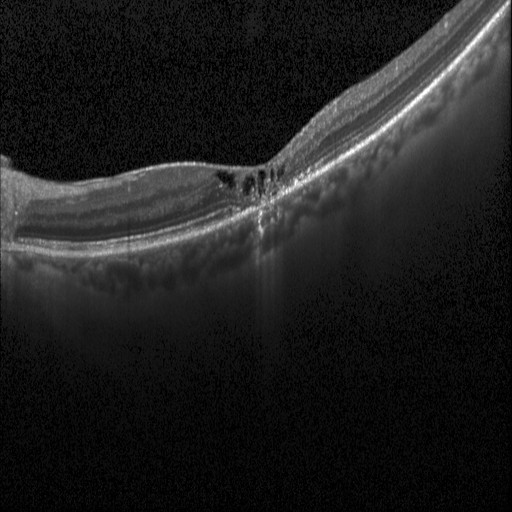 Optical coherence tomography scan. Spectral-domain optical coherence tomography. Heidelberg Spectralis OCT system. Centered on the fovea
This B-scan demonstrates diabetic macular edema (DME).